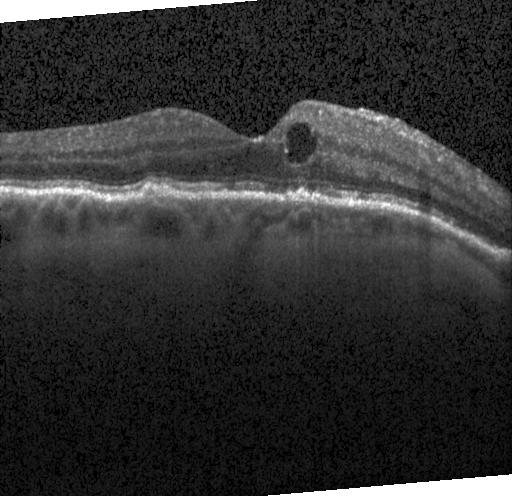 Horizontal scan through the fovea. Heidelberg Spectralis OCT system. SD-OCT. Retinal OCT B-scan. OCT finding: CNV.